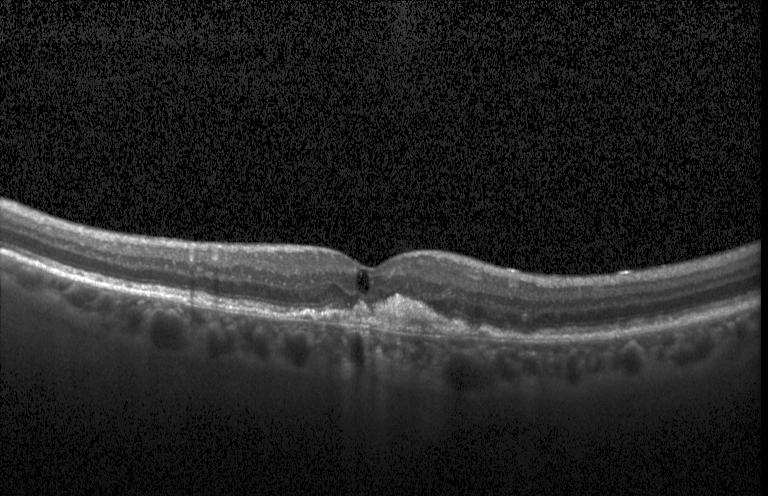

Instrument: Heidelberg Spectralis, spectral-domain OCT, optical coherence tomography scan
Assessment: a choroidal neovascular membrane.